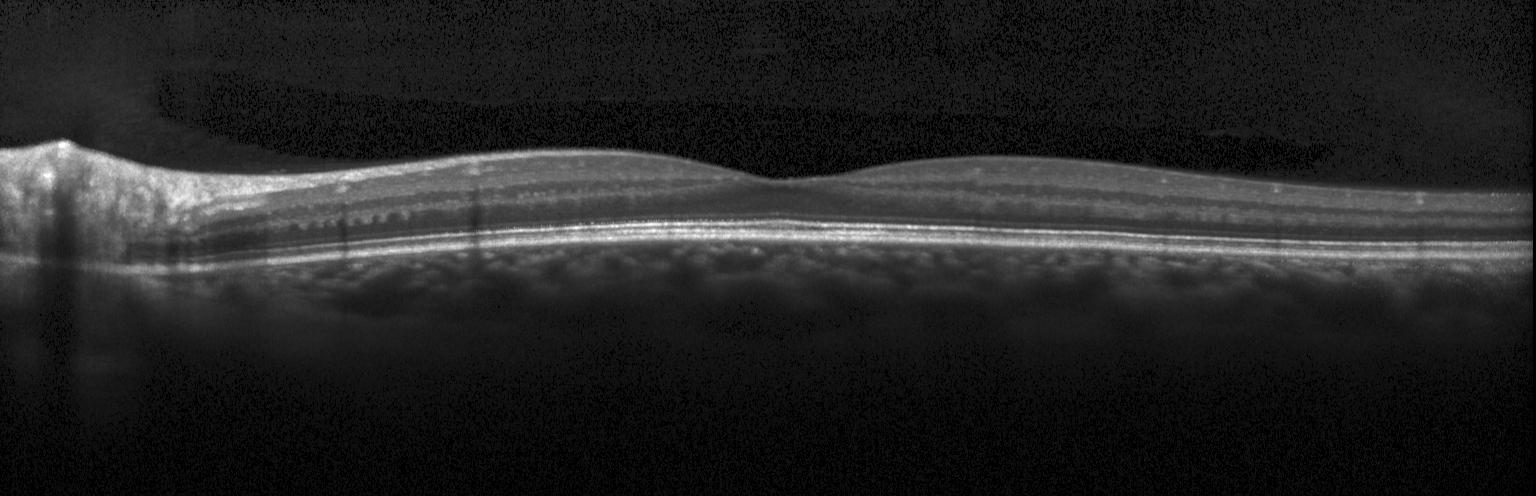 The scan shows no choroidal neovascularization, no diabetic macular edema, and no drusen.